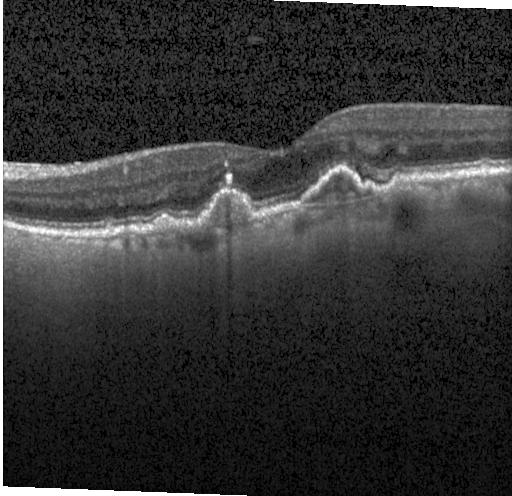

Heidelberg Spectralis, OCT line scan
A choroidal neovascular membrane.